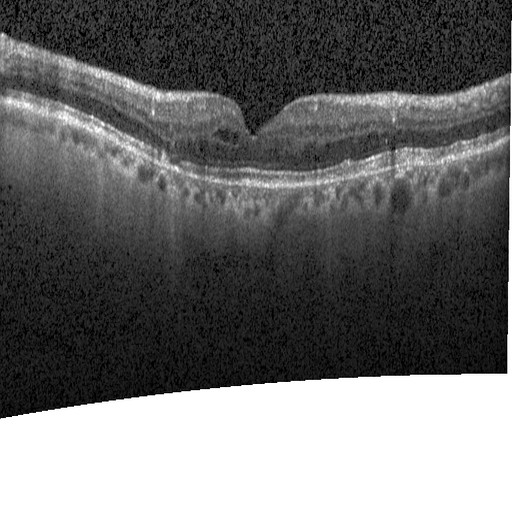 Optical coherence tomography scan
Diagnosis: DME.